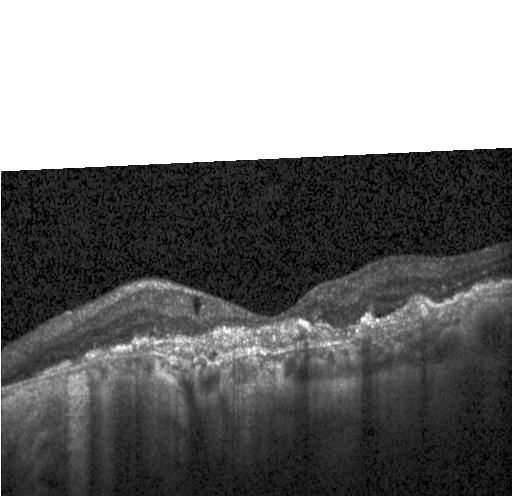
Assessment: choroidal neovascularization.